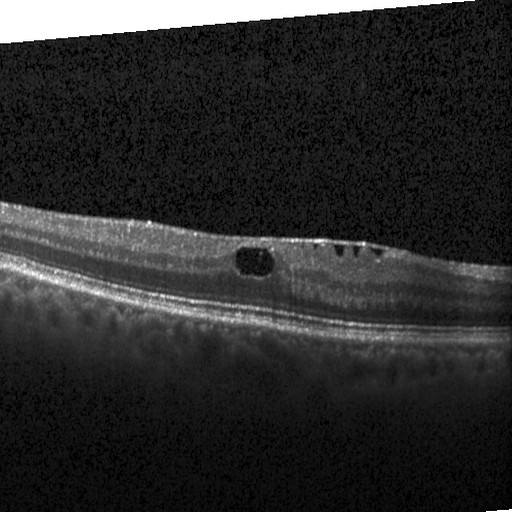

Retinal OCT cross-section. Macular scan. SD-OCT. Macular OCT: DME.